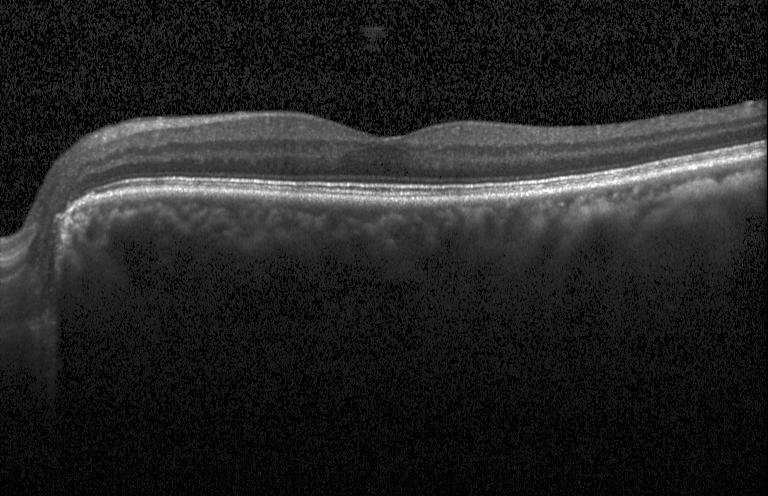

Instrument: Heidelberg Spectralis · retinal OCT cross-section — Dx: neither choroidal neovascularization, diabetic macular edema, nor drusen.